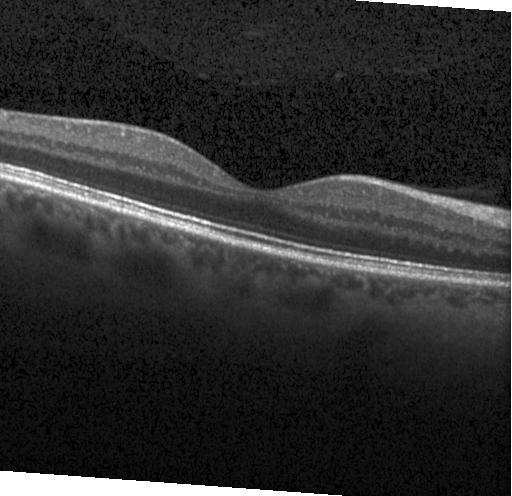
Finding: no choroidal neovascularization, diabetic macular edema, or drusen.